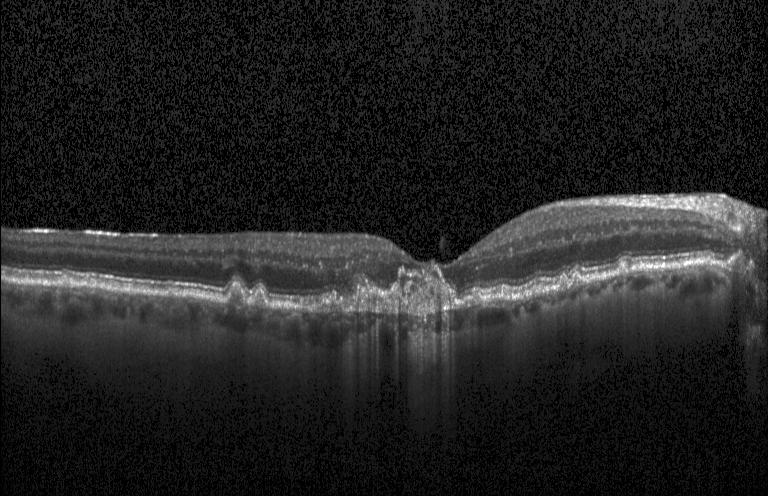
Spectral-domain OCT · instrument: Heidelberg Spectralis · OCT B-scan — OCT finding: a choroidal neovascular membrane.